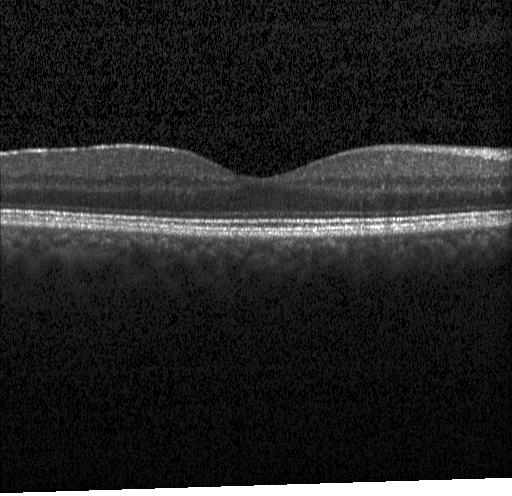 SD-OCT, Heidelberg Spectralis OCT system, macular scan, optical coherence tomography scan. Diagnosis: no choroidal neovascularization, no diabetic macular edema, and no drusen.